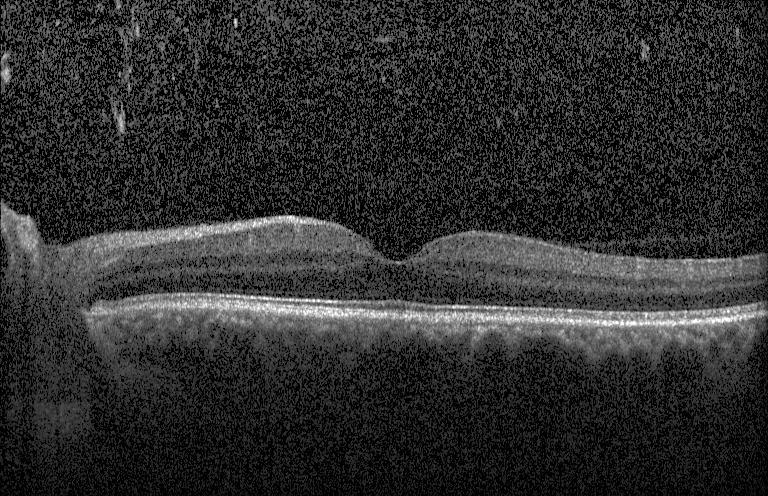 Optical coherence tomography B-scan · spectral-domain optical coherence tomography.
Diagnosis: neither choroidal neovascularization, diabetic macular edema, nor drusen.